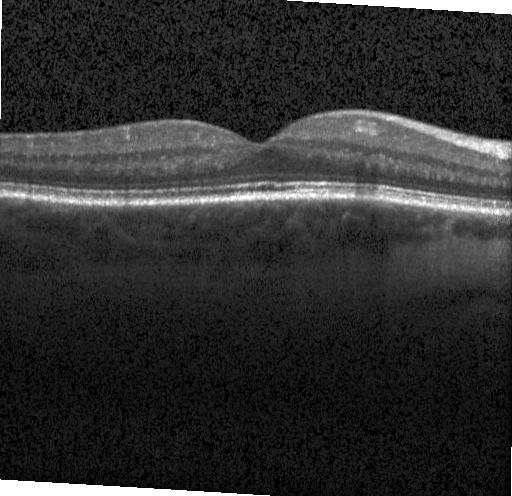

Impression: no evidence of CNV, DME, or drusen.